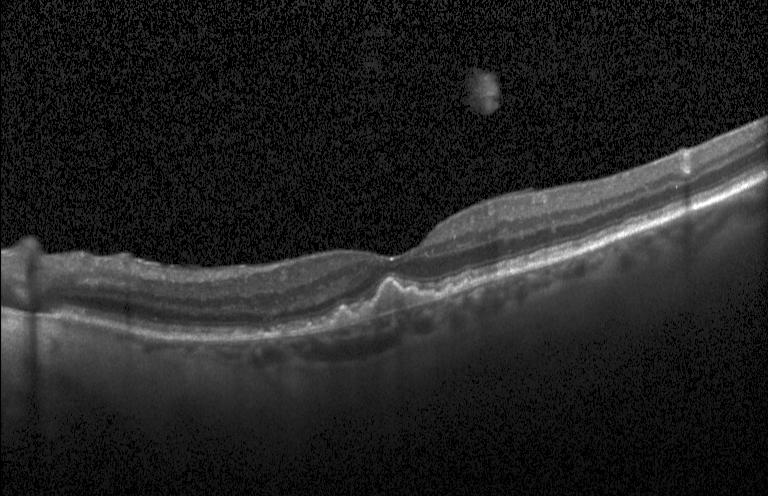

OCT finding: multiple drusen.